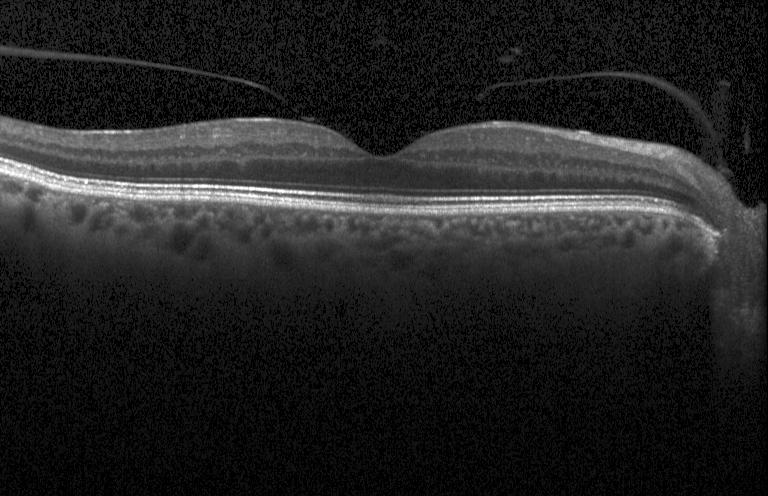
OCT line scan. The scan shows no choroidal neovascularization, no diabetic macular edema, and no drusen.